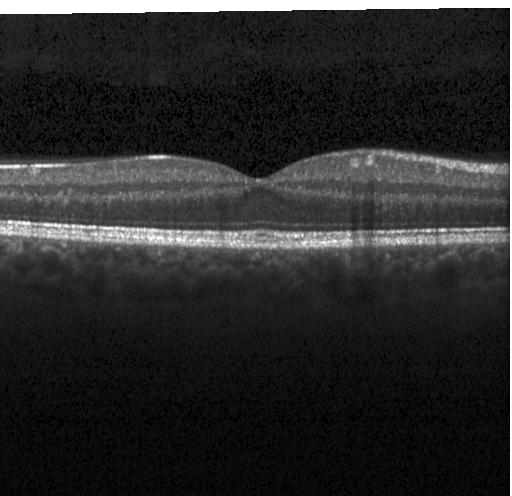

Retinal OCT B-scan
Dx: no evidence of choroidal neovascularization, diabetic macular edema, or drusen.